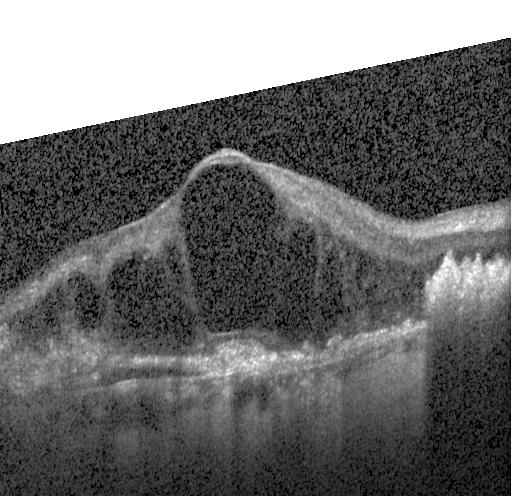
Retinal OCT cross-section showing a choroidal neovascular membrane.